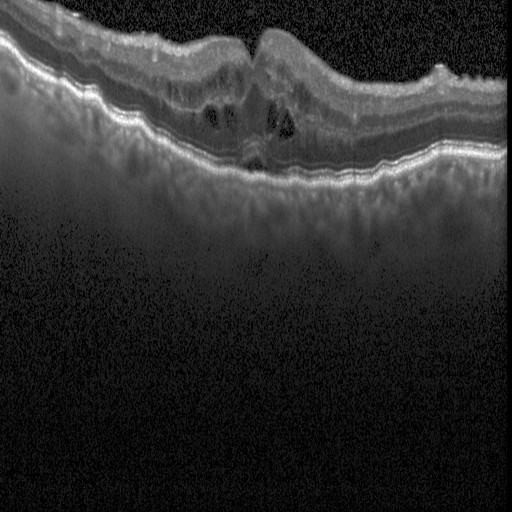

Through the macula, OCT B-scan, spectral-domain OCT — Assessment: diabetic macular edema.